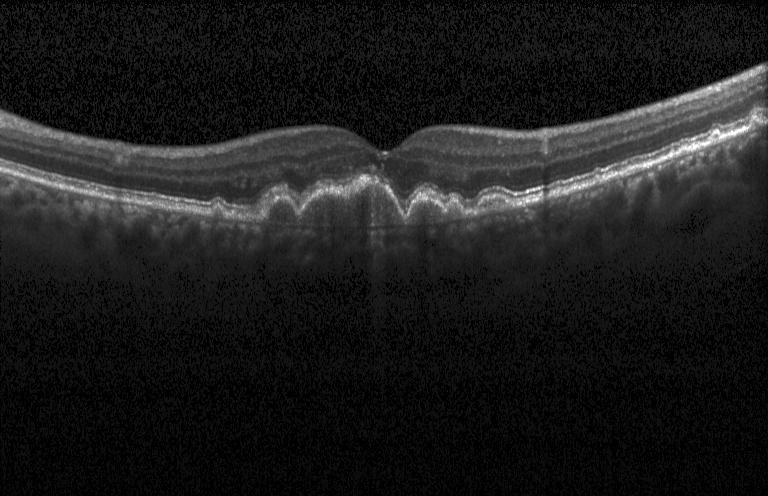

Retinal OCT cross-section · macular scan · spectral-domain optical coherence tomography. Diagnosis: drusen.